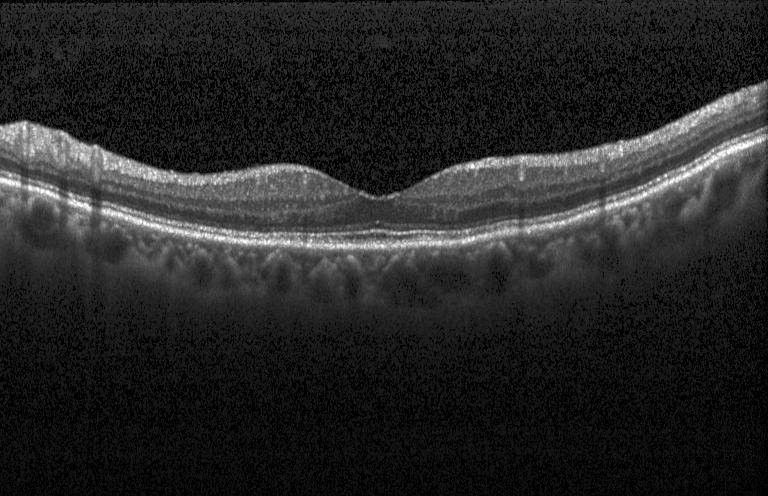

Instrument: Heidelberg Spectralis, OCT B-scan. OCT finding: neither choroidal neovascularization, diabetic macular edema, nor drusen.